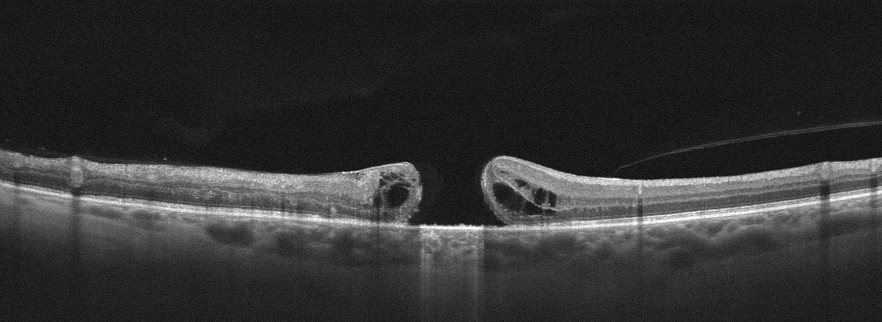
Oculus dexter, optical coherence tomography B-scan
Impression: vitreomacular interface disease (VID).